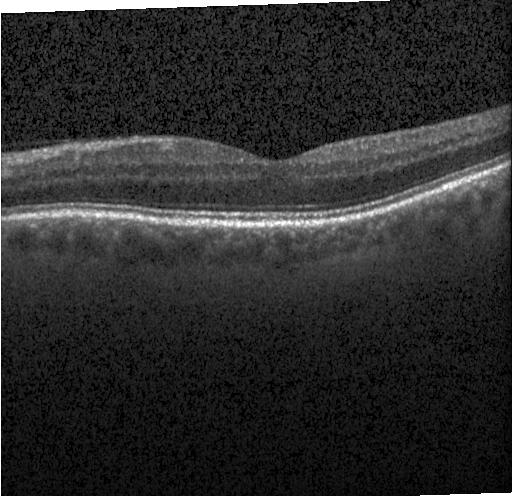
Centered on the fovea, optical coherence tomography scan, spectral-domain optical coherence tomography, acquired on a Heidelberg Spectralis.
Impression: no CNV, DME, or drusen.